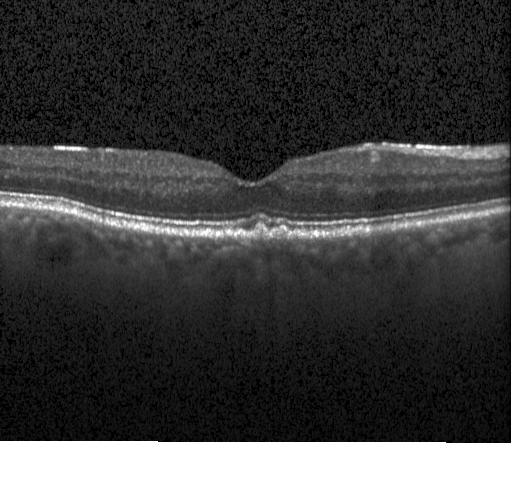 Retinal OCT B-scan
Diagnosis: sub-RPE drusenoid deposits.